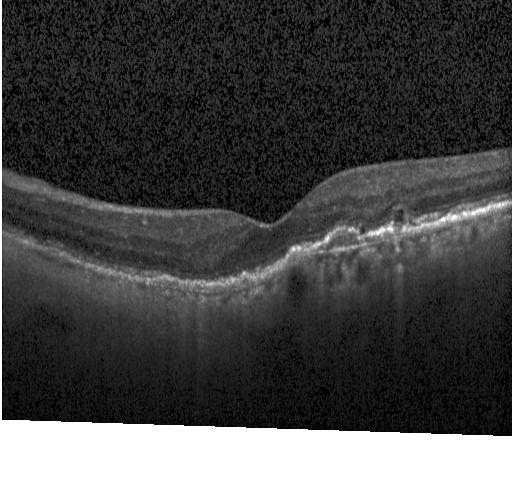
Spectral-domain OCT; macular scan; retinal OCT cross-section. Impression: a choroidal neovascular membrane.